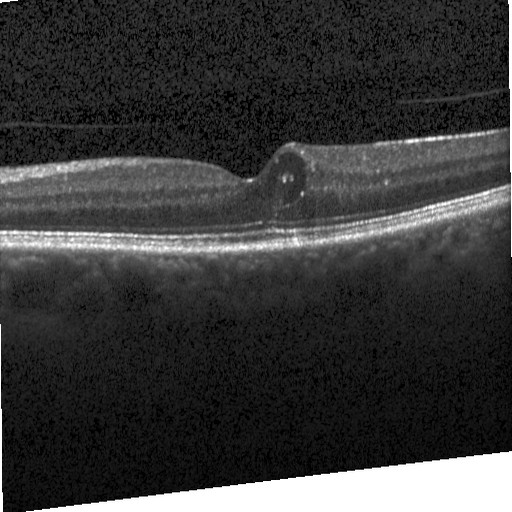 Optical coherence tomography B-scan; instrument: Heidelberg Spectralis; macular scan. Diagnosis: DME.